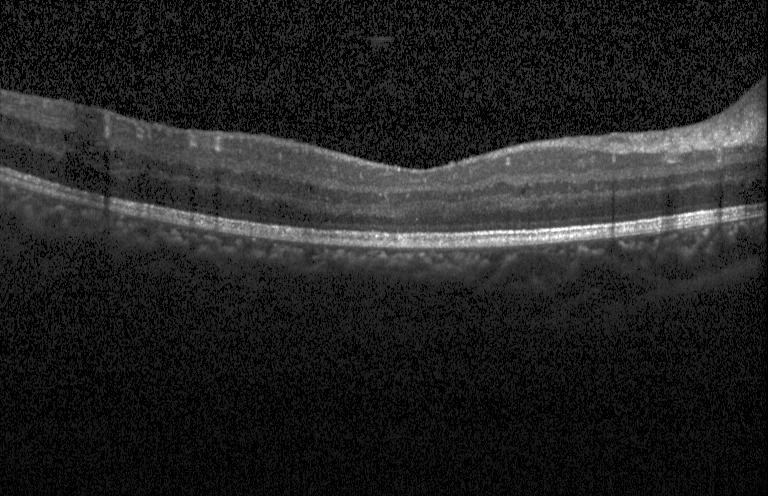
Retinal OCT cross-section showing no CNV, no DME, and no drusen.